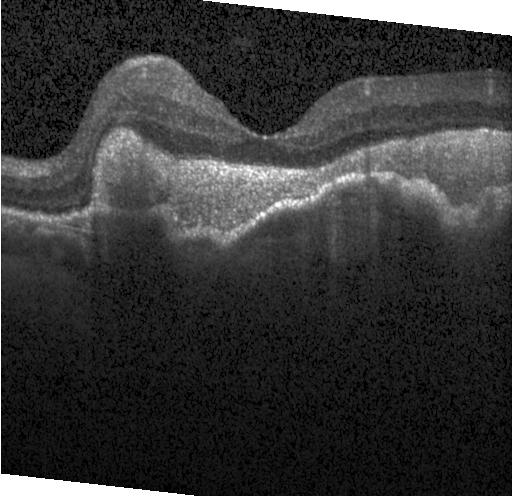 Spectral-domain optical coherence tomography · through the macula · Heidelberg Spectralis · retinal OCT cross-section.
Diagnosis: choroidal neovascularization (CNV).